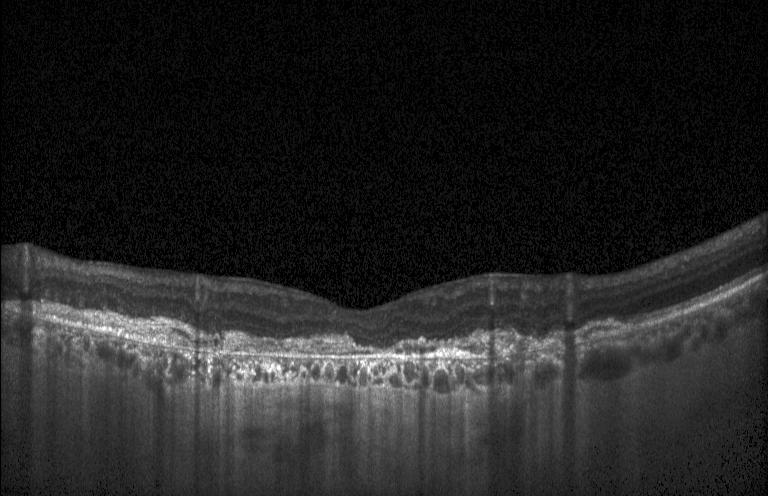

OCT finding: CNV.